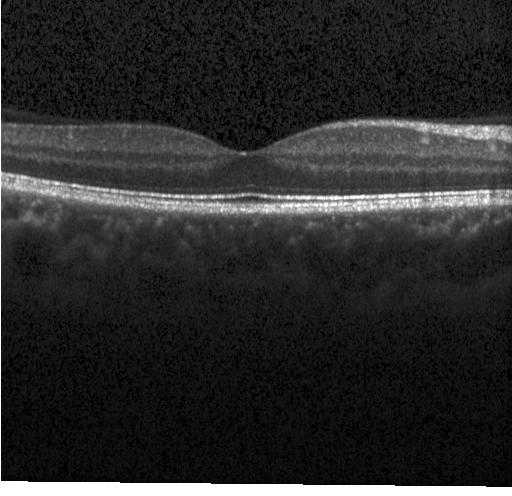 Impression: no evidence of choroidal neovascularization, diabetic macular edema, or drusen.